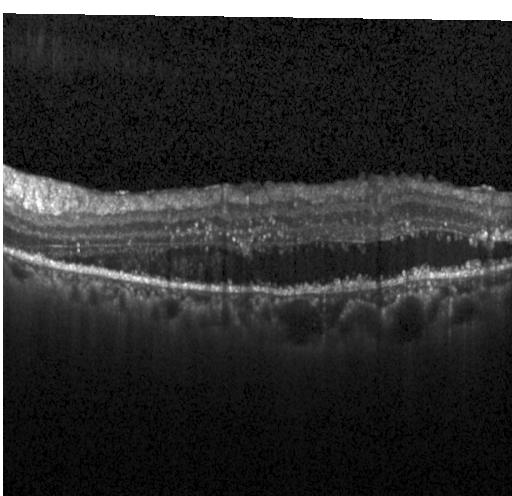 Retinal OCT cross-section · instrument: Heidelberg Spectralis.
OCT finding: a choroidal neovascular membrane.